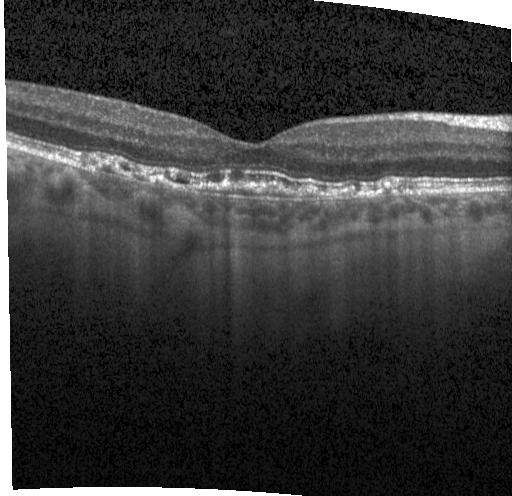 Diagnosis: choroidal neovascularization (CNV).